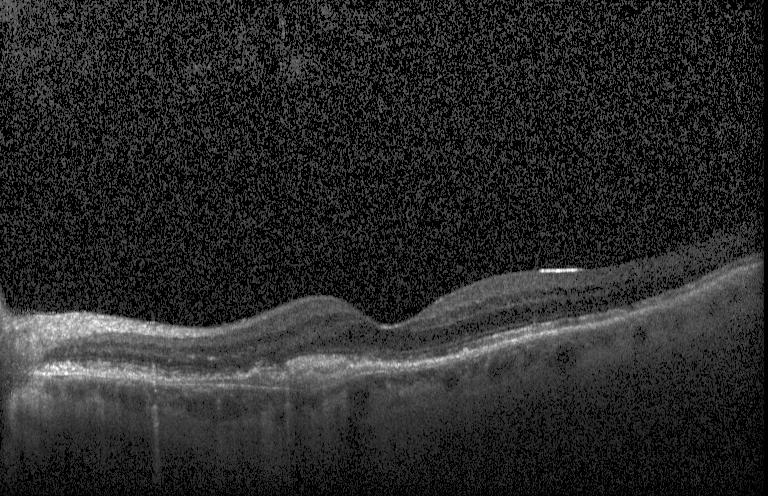 Dx: a choroidal neovascular membrane.